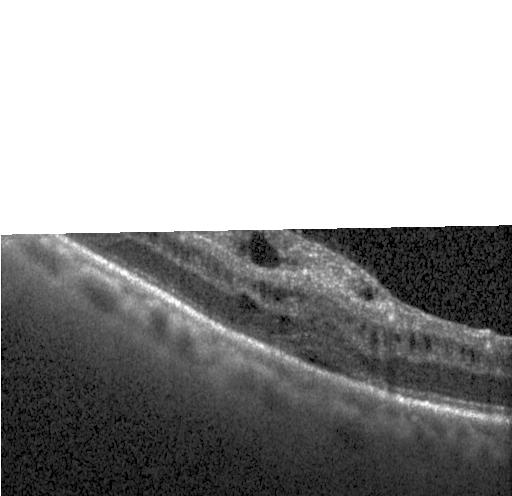
Heidelberg Spectralis OCT system, OCT B-scan, spectral-domain OCT, macular scan. Assessment: diabetic macular edema.